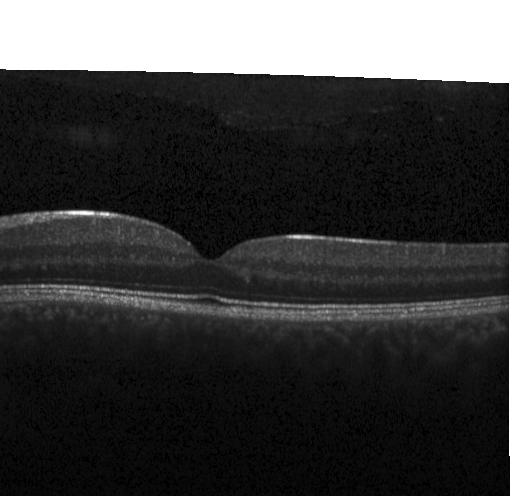 Impression: neither choroidal neovascularization, diabetic macular edema, nor drusen.